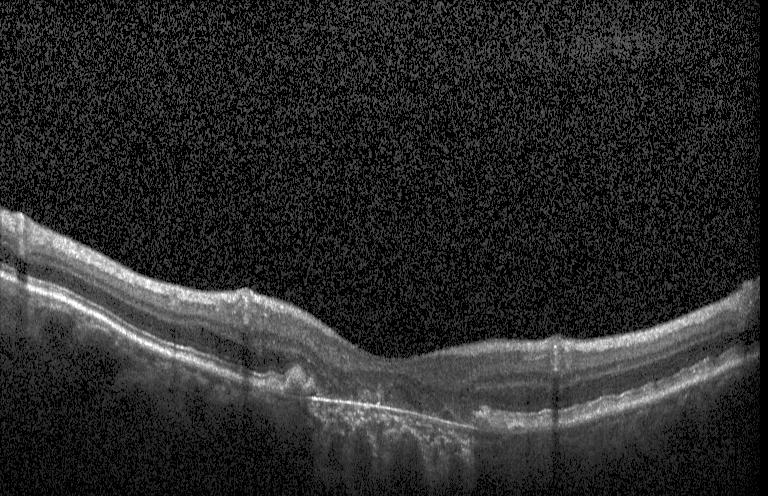
The scan shows choroidal neovascularization (CNV).